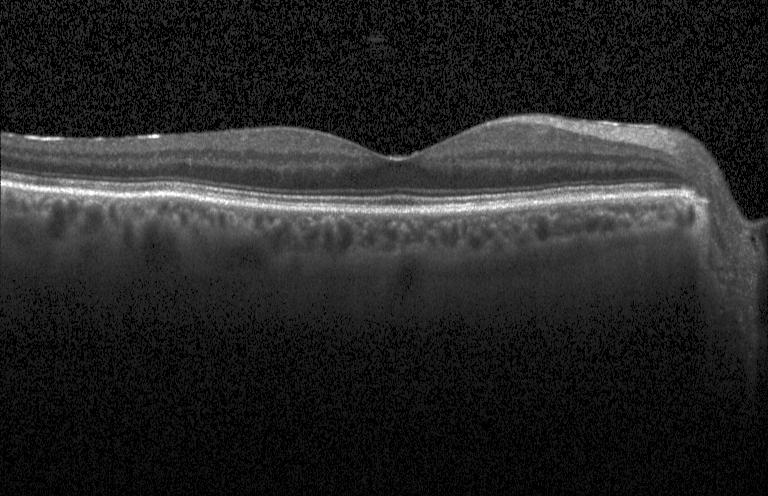
Finding: no evidence of choroidal neovascularization, diabetic macular edema, or drusen.